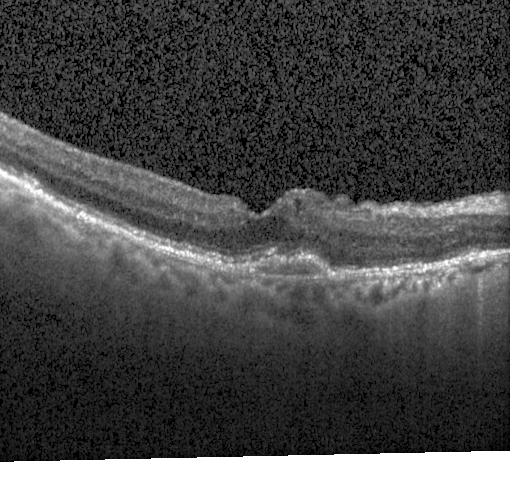 Spectral-domain optical coherence tomography, acquired on a Heidelberg Spectralis, horizontal scan through the fovea, retinal OCT B-scan
This B-scan demonstrates choroidal neovascularization.